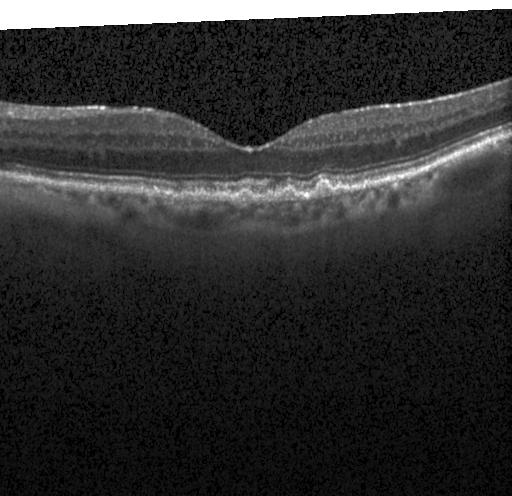

Heidelberg Spectralis; centered on the fovea; spectral-domain optical coherence tomography; optical coherence tomography scan
Impression: drusen.